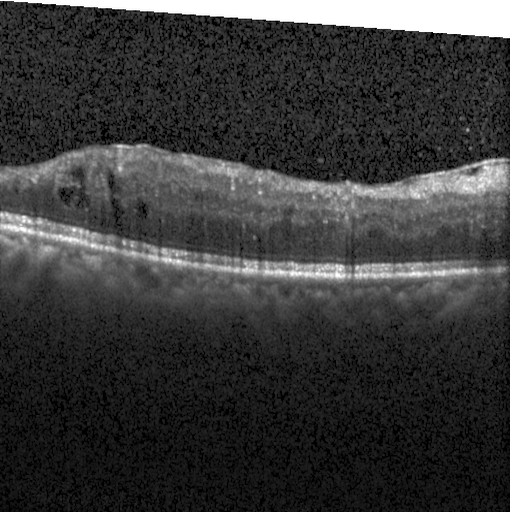
Dx: diabetic macular edema (DME).